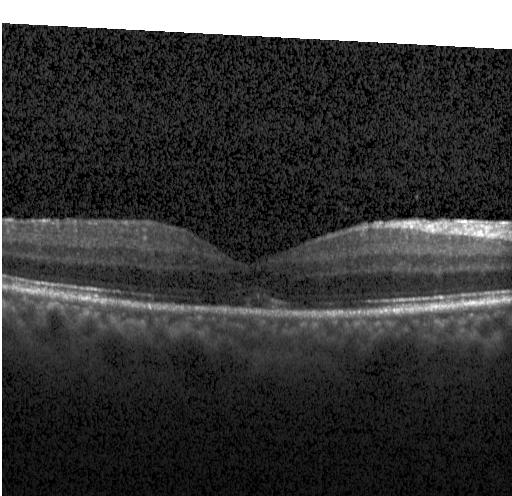
Horizontal scan through the fovea · optical coherence tomography B-scan · spectral-domain OCT · instrument: Heidelberg Spectralis. This B-scan demonstrates neither CNV, DME, nor drusen.